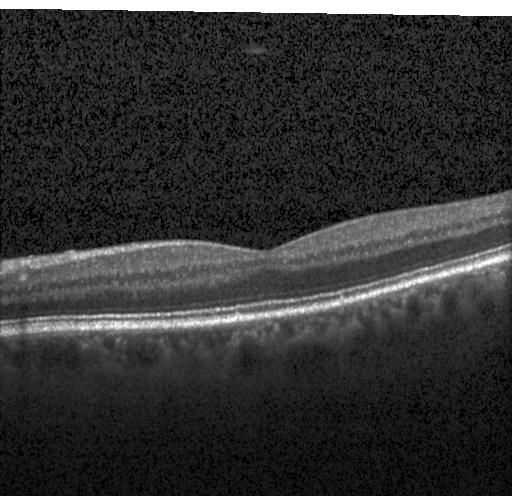 Diagnosis: no CNV, no DME, and no drusen.